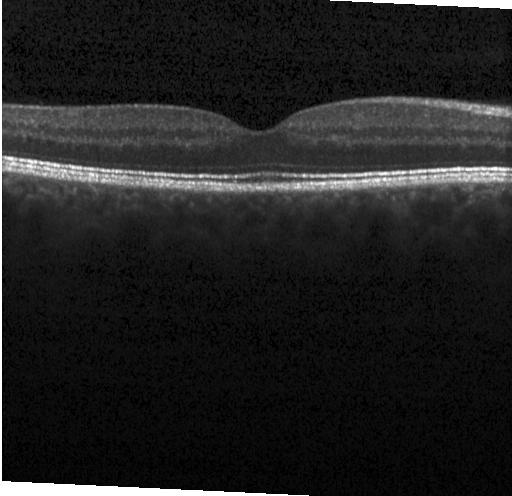 The scan shows neither choroidal neovascularization, diabetic macular edema, nor drusen.